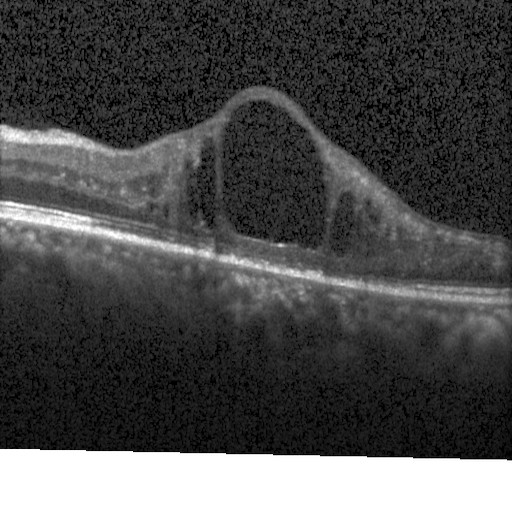 Finding: diabetic macular edema (DME).